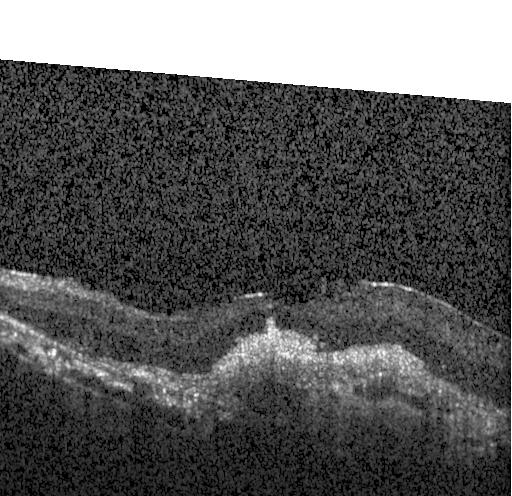

Finding: CNV.